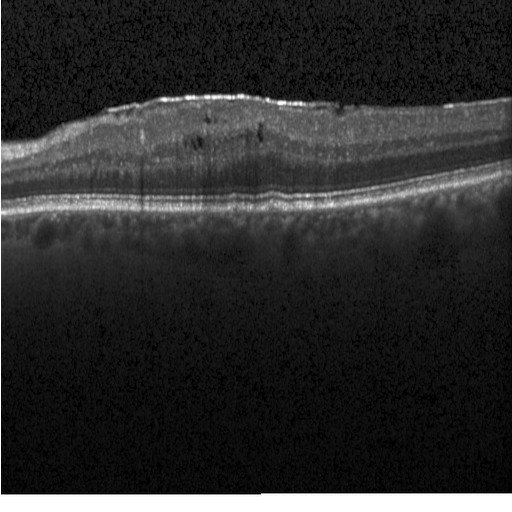 Retinal OCT cross-section. Spectral-domain OCT. Heidelberg Spectralis
Macular OCT: diabetic macular edema.